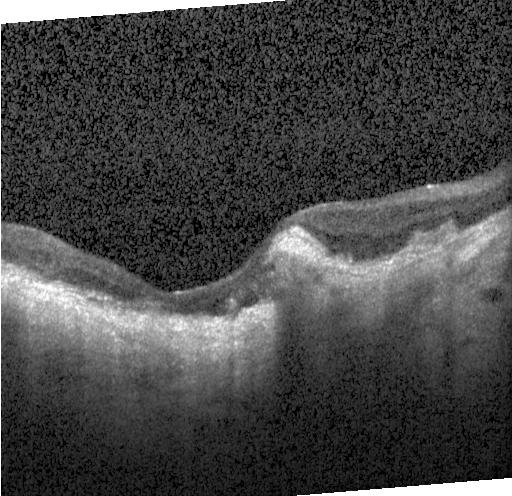
Retinal OCT B-scan — This B-scan demonstrates a choroidal neovascular membrane.